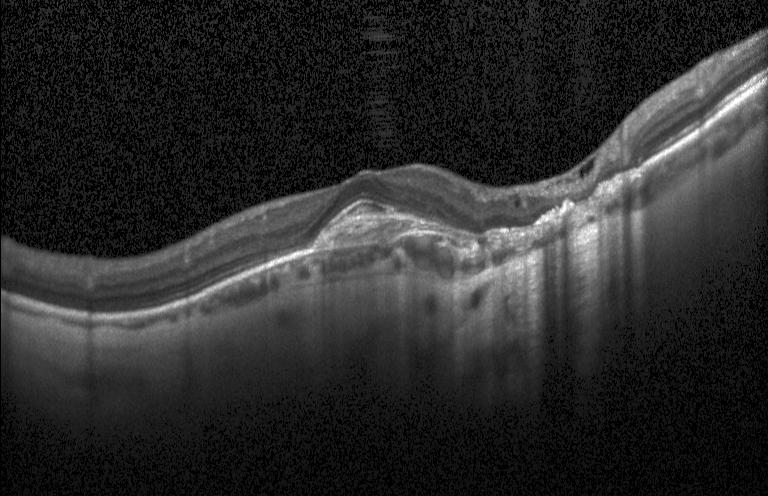
Macular scan · retinal OCT cross-section
OCT finding: CNV.